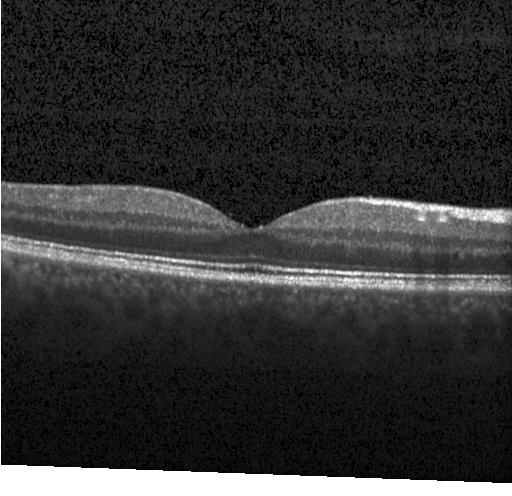 Diagnosis: no evidence of choroidal neovascularization, diabetic macular edema, or drusen.